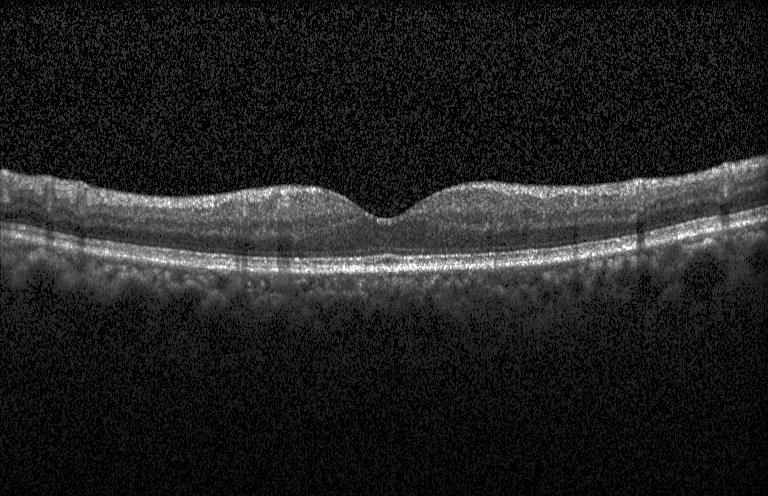
SD-OCT. OCT line scan. Assessment: no choroidal neovascularization, no diabetic macular edema, and no drusen.